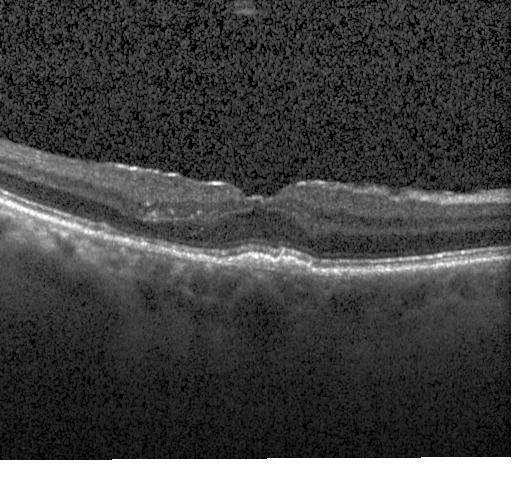

OCT line scan
Dx: choroidal neovascularization.